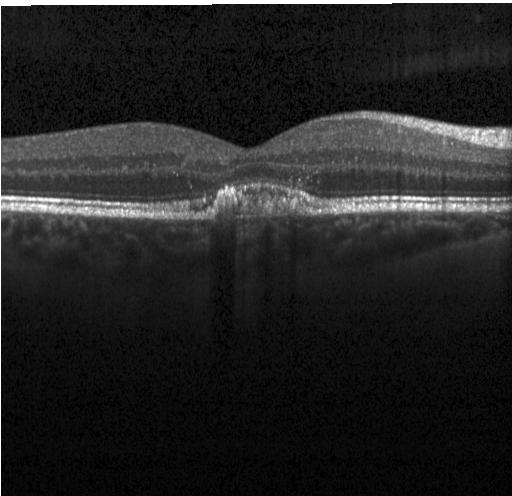 Heidelberg Spectralis · OCT line scan — Diagnosis: a choroidal neovascular membrane.